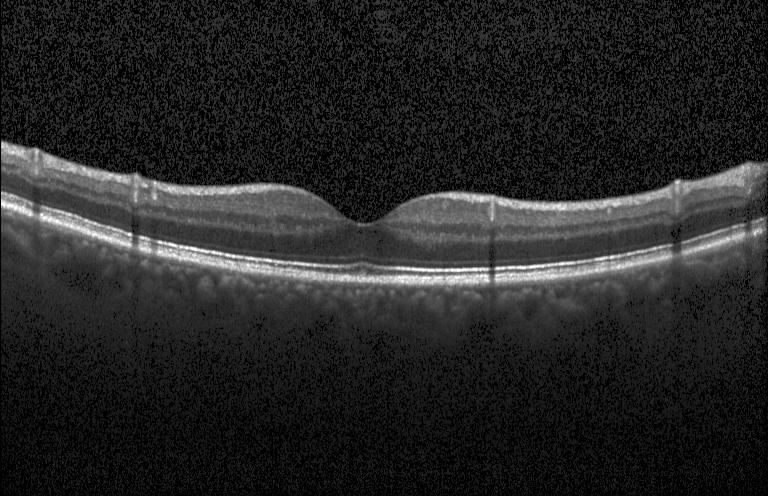

OCT B-scan — Assessment: no CNV, DME, or drusen.